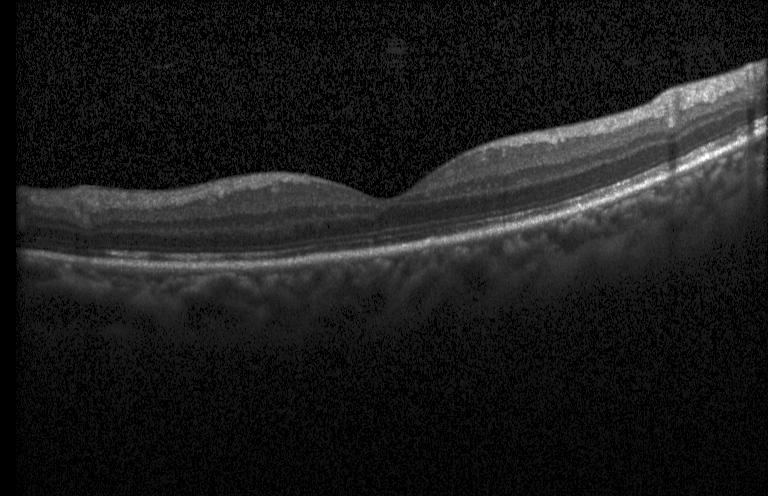 Dx: no CNV, no DME, and no drusen.